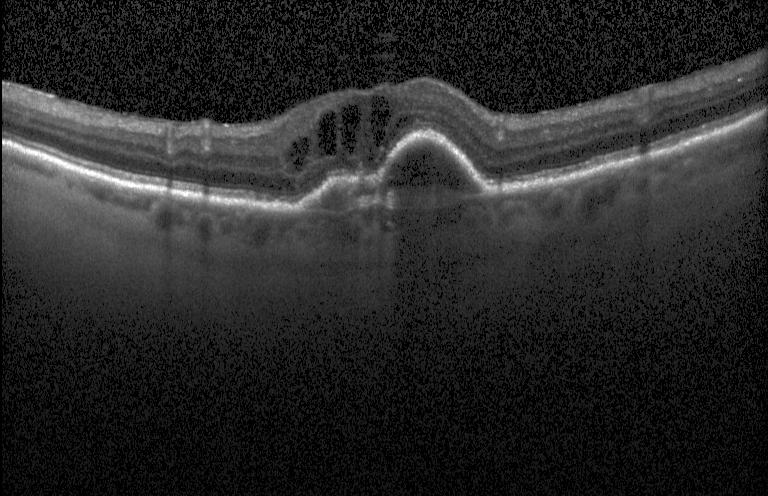

OCT scan showing choroidal neovascularization (CNV).